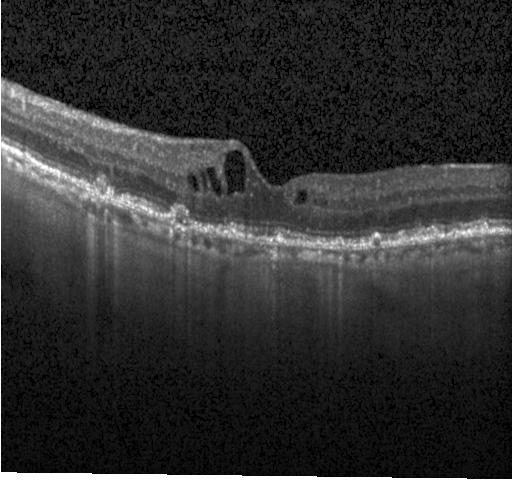

Spectral-domain OCT, horizontal scan through the fovea, Heidelberg Spectralis OCT system, optical coherence tomography B-scan
Assessment: a choroidal neovascular membrane.